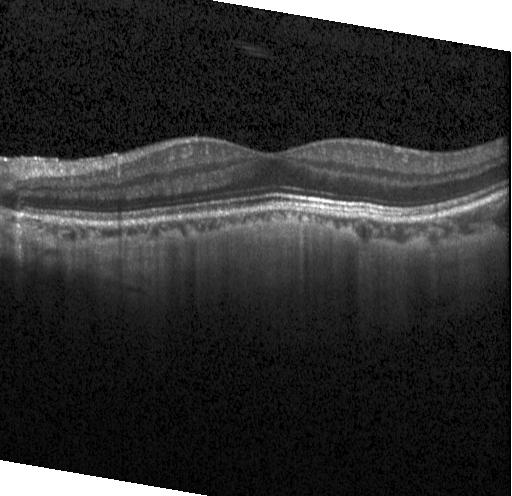
Spectral-domain OCT B-scan: neither choroidal neovascularization, diabetic macular edema, nor drusen.